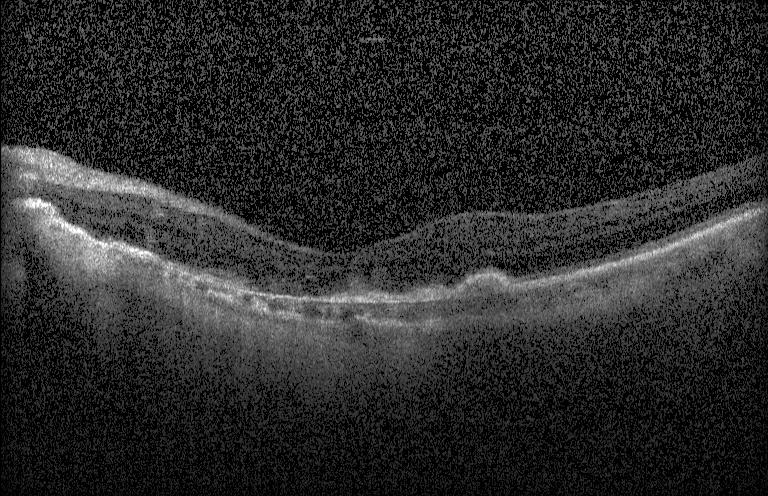 Retinal OCT B-scan. Dx: choroidal neovascularization.